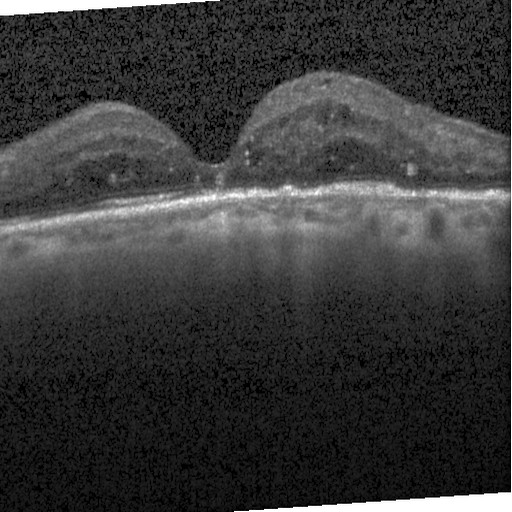 Assessment: diabetic macular edema (DME).